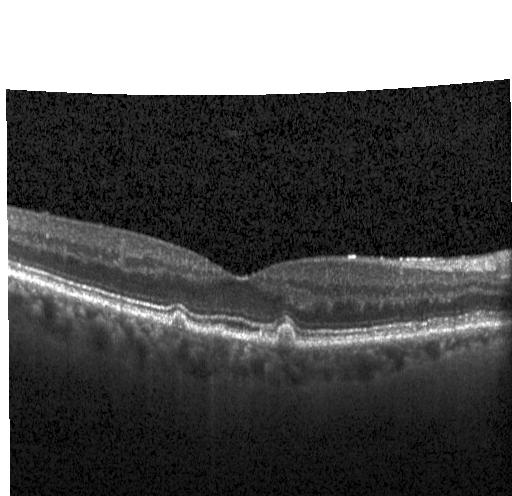
Heidelberg Spectralis; spectral-domain OCT; fovea-centered; OCT line scan. Sub-RPE drusenoid deposits.